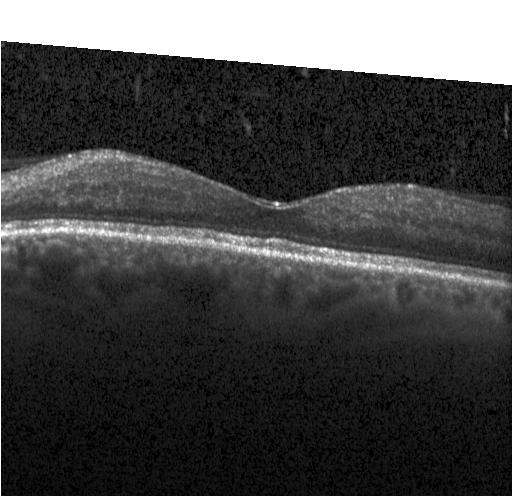 Optical coherence tomography scan; spectral-domain OCT; centered on the fovea — The scan shows neither choroidal neovascularization, diabetic macular edema, nor drusen.